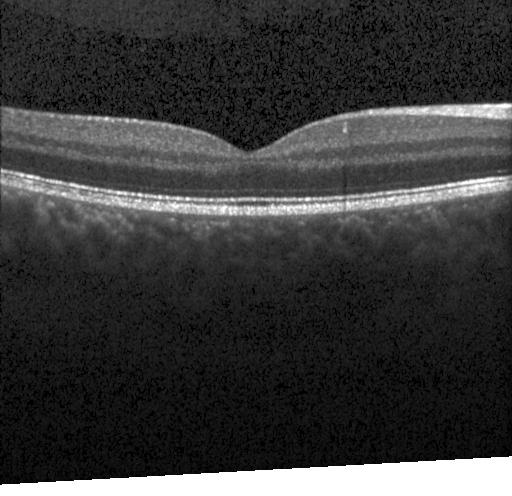 SD-OCT, Heidelberg Spectralis OCT system, OCT B-scan — Finding: neither choroidal neovascularization, diabetic macular edema, nor drusen.